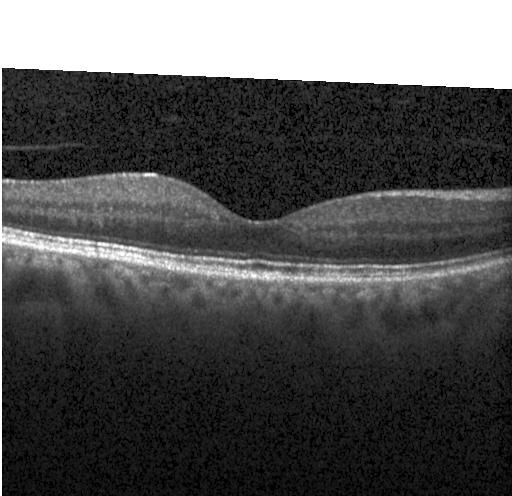
Horizontal scan through the fovea; acquired on a Heidelberg Spectralis; optical coherence tomography scan; spectral-domain OCT. Assessment: no choroidal neovascularization, diabetic macular edema, or drusen.